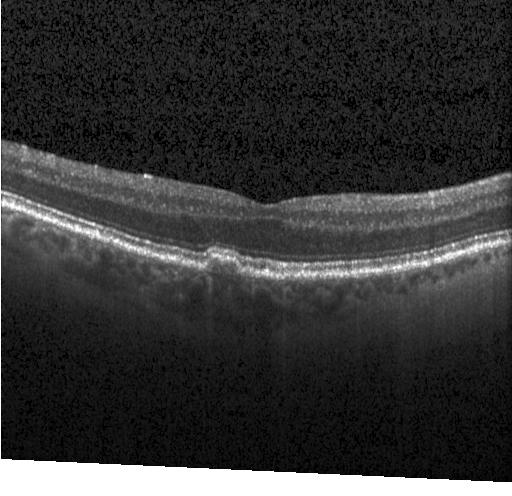

Heidelberg Spectralis; SD-OCT; retinal OCT cross-section
OCT finding: drusen.